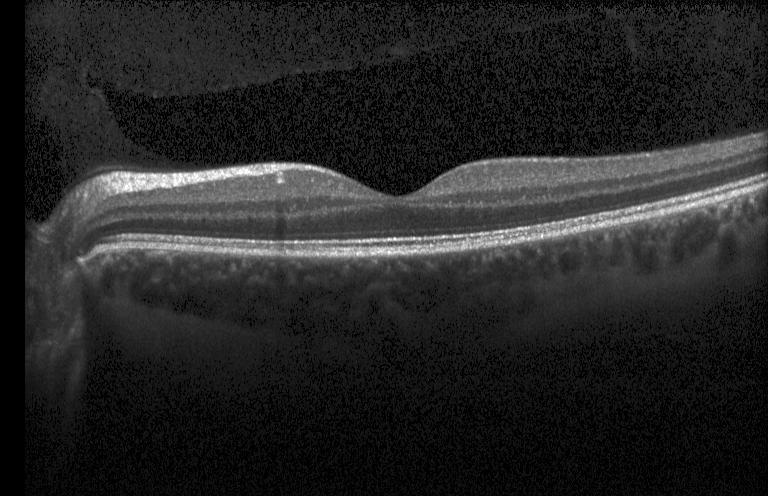
Diagnosis: no evidence of choroidal neovascularization, diabetic macular edema, or drusen.